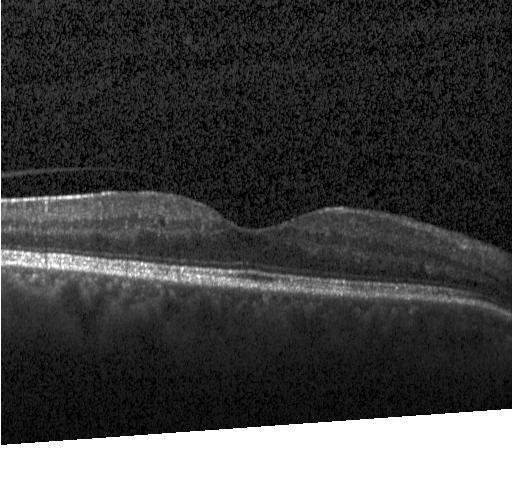 Retinal OCT cross-section showing no CNV, DME, or drusen.